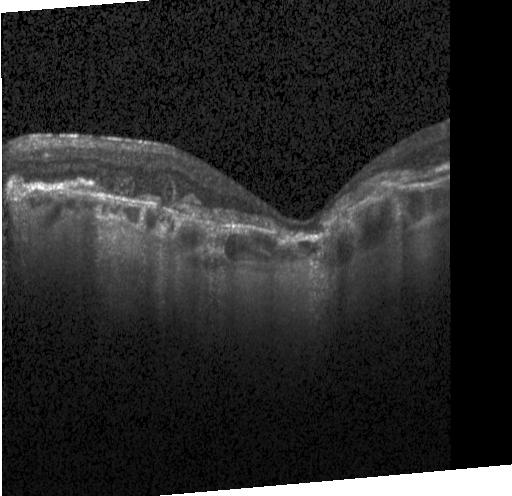 Spectral-domain OCT B-scan: CNV.